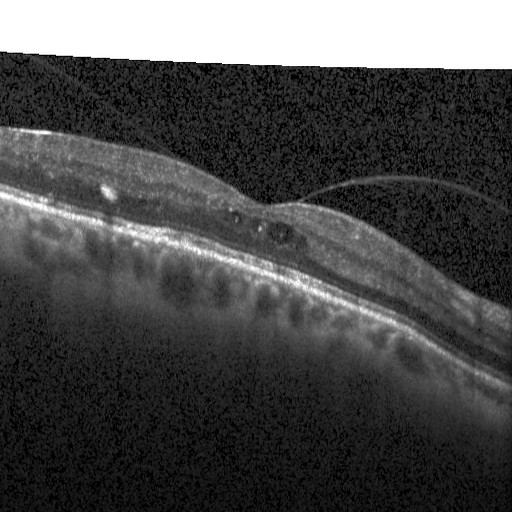

OCT line scan; spectral-domain OCT; through the macula. Finding: diabetic macular edema.